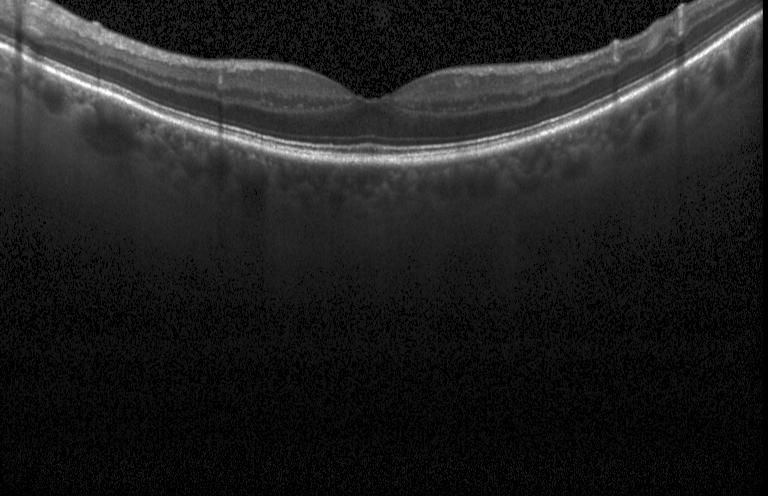 Dx: neither choroidal neovascularization, diabetic macular edema, nor drusen.